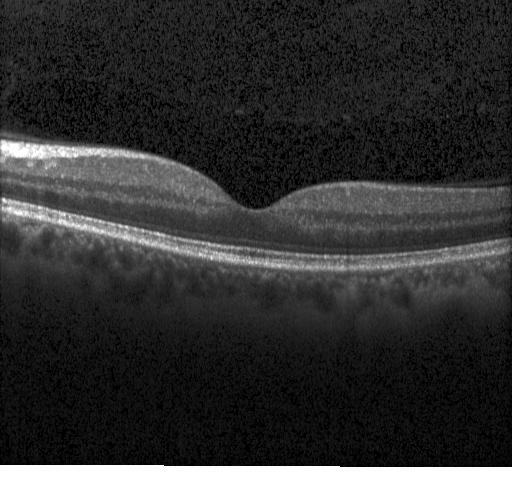
Heidelberg Spectralis OCT system, optical coherence tomography B-scan, horizontal scan through the fovea. OCT finding: no evidence of choroidal neovascularization, diabetic macular edema, or drusen.